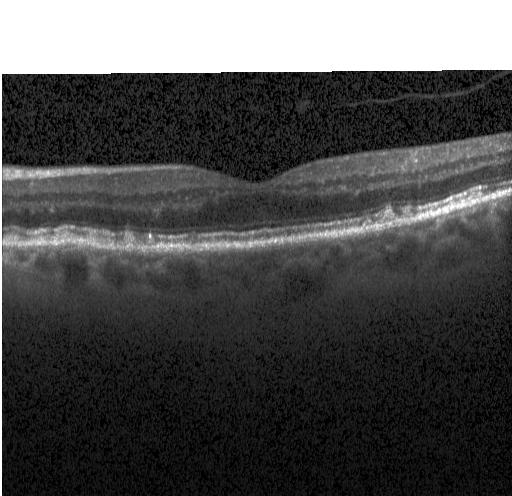
Impression: sub-RPE drusenoid deposits.